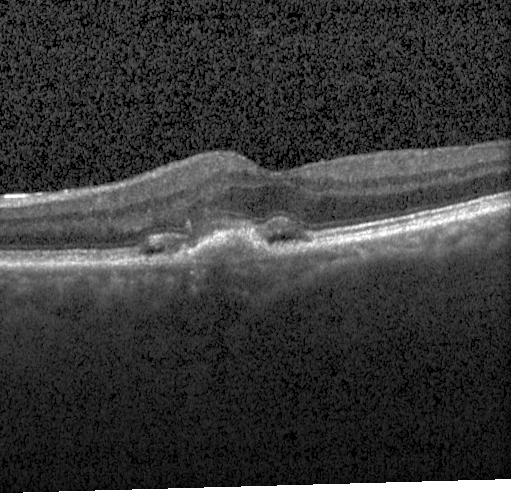 Acquired on a Heidelberg Spectralis. OCT B-scan. Finding: choroidal neovascularization (CNV).